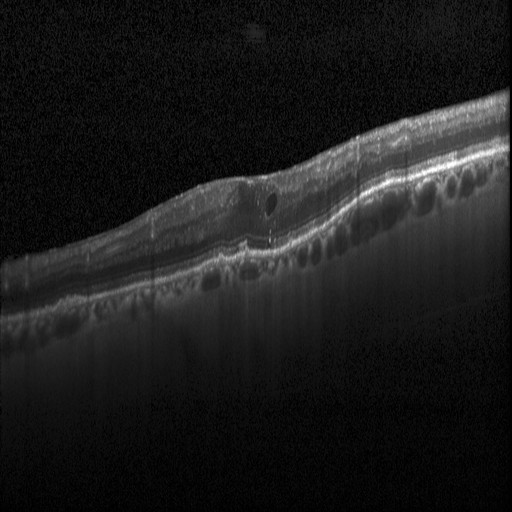
OCT line scan; spectral-domain optical coherence tomography; horizontal scan through the fovea; instrument: Heidelberg Spectralis.
Impression: DME.